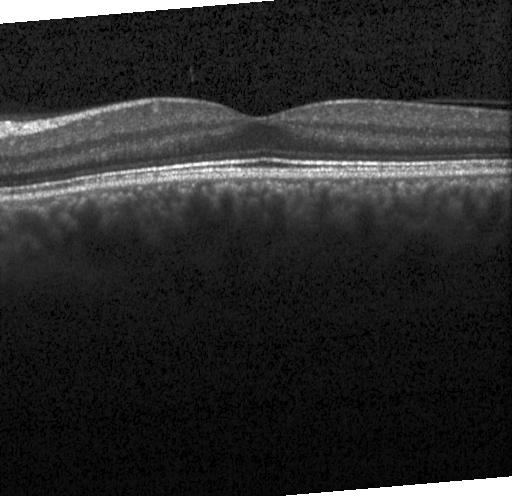

Retinal OCT B-scan. Finding: neither choroidal neovascularization, diabetic macular edema, nor drusen.